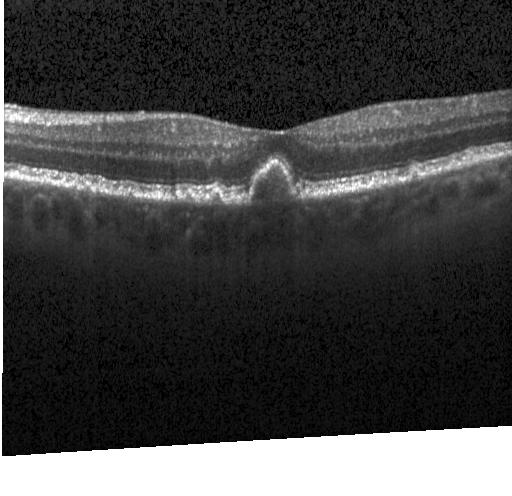

Retinal OCT B-scan; spectral-domain optical coherence tomography; instrument: Heidelberg Spectralis — Finding: multiple drusen.